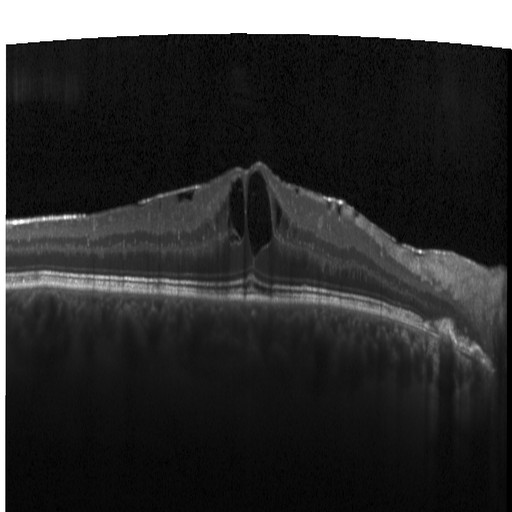 Optical coherence tomography B-scan. Finding: diabetic macular edema (DME).